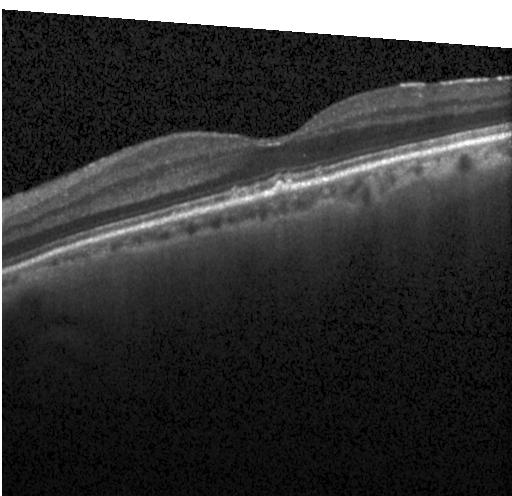

Retinal OCT cross-section — Impression: drusen.